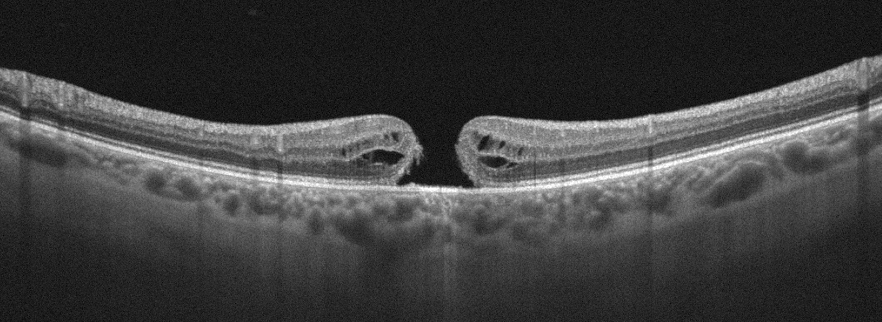 Retinal OCT B-scan, oculus dexter.
Impression: VID.